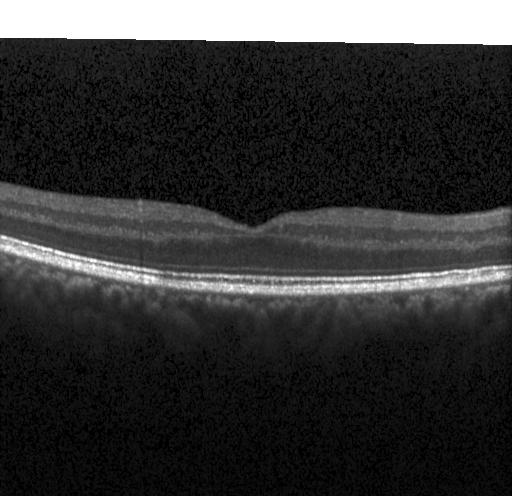

Optical coherence tomography B-scan.
Impression: no evidence of choroidal neovascularization, diabetic macular edema, or drusen.